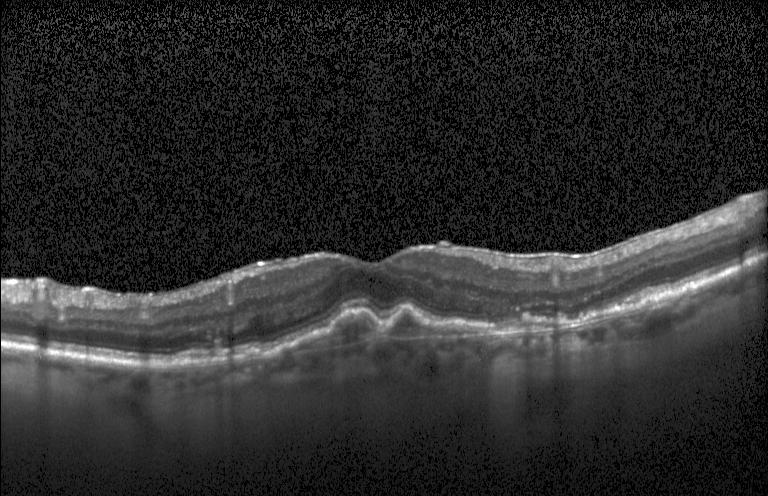
This B-scan demonstrates choroidal neovascularization (CNV).